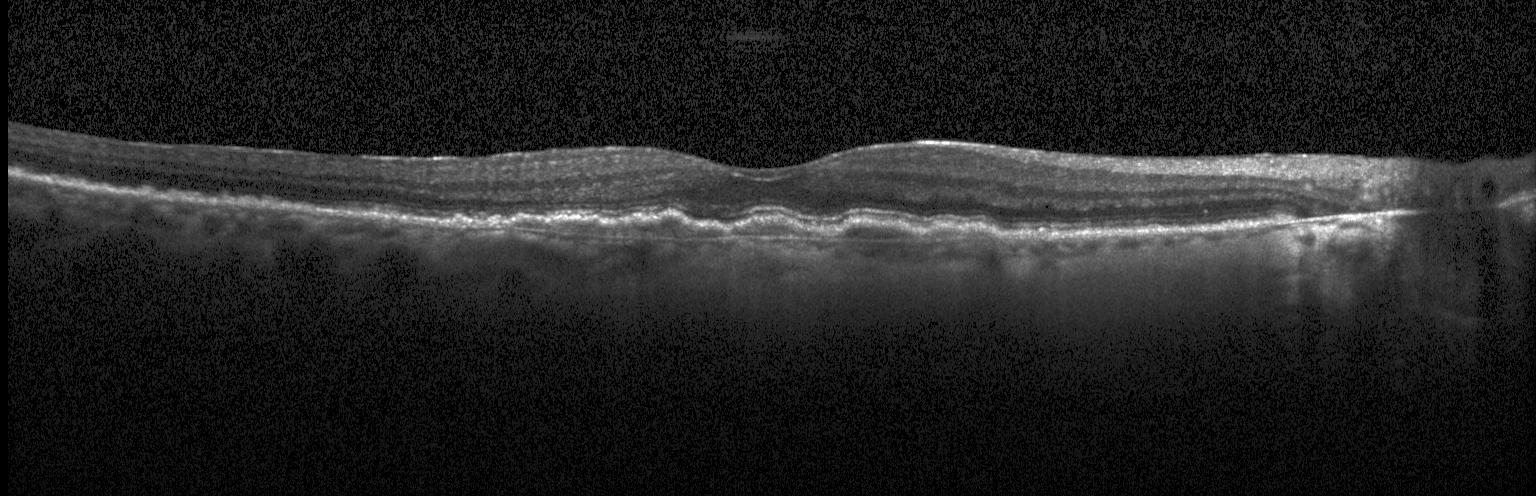
Retinal OCT cross-section — Impression: choroidal neovascularization.